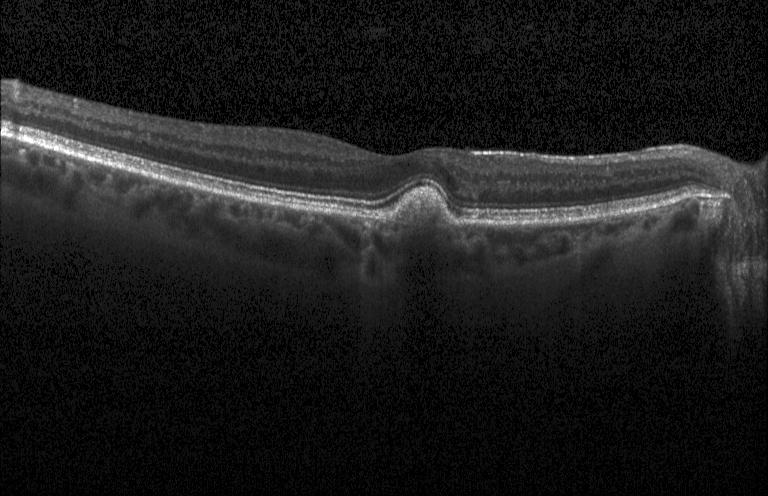 OCT scan showing sub-RPE drusenoid deposits.